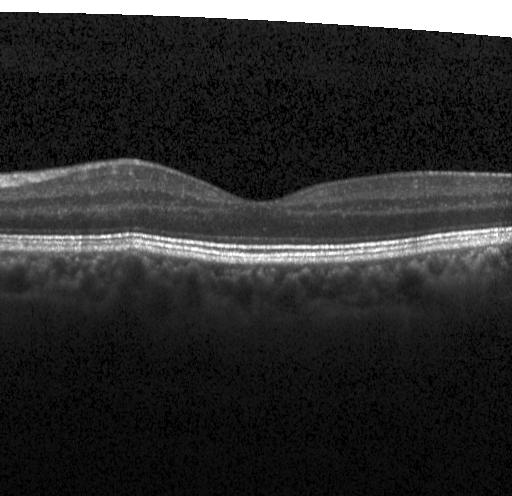 Macular OCT demonstrating no choroidal neovascularization, diabetic macular edema, or drusen.